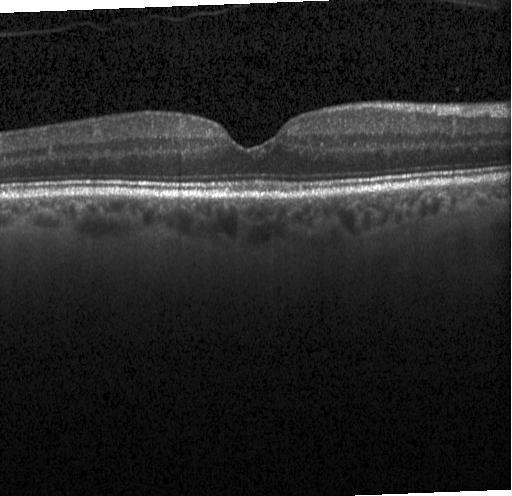
Finding: no evidence of choroidal neovascularization, diabetic macular edema, or drusen.